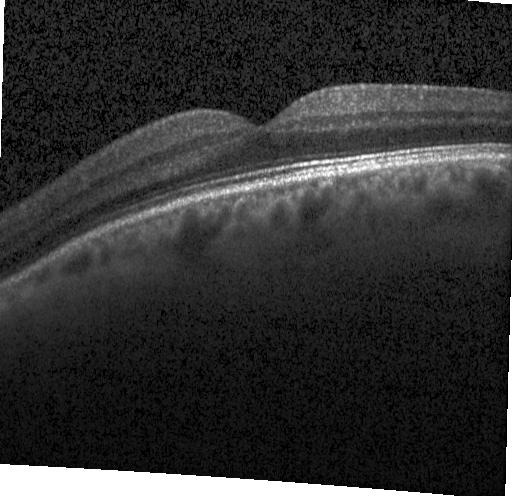
Diagnosis: no evidence of CNV, DME, or drusen.